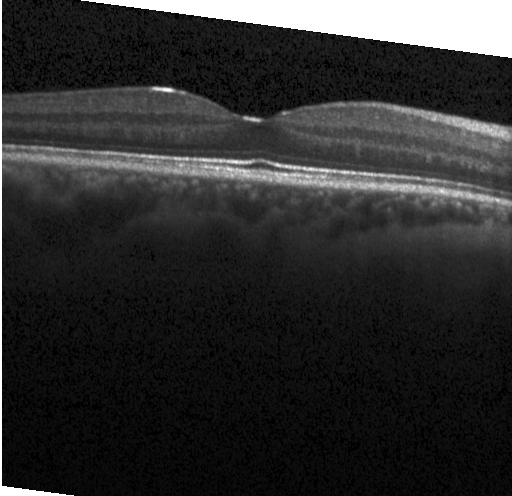 Spectral-domain optical coherence tomography, instrument: Heidelberg Spectralis, optical coherence tomography B-scan, horizontal scan through the fovea — Impression: no CNV, DME, or drusen.